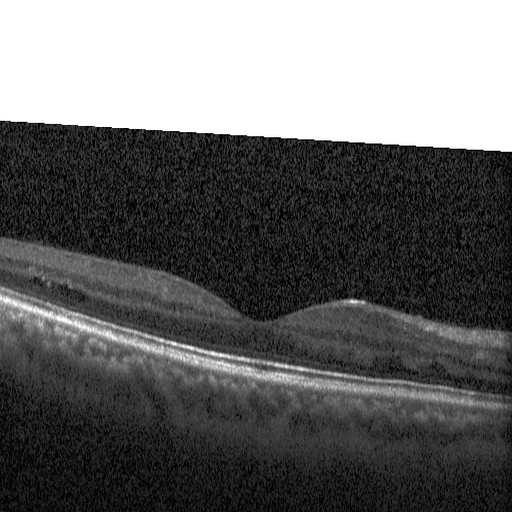
Finding: diabetic macular edema.